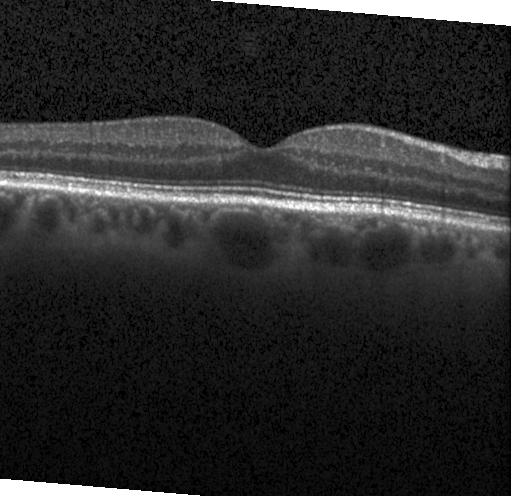

Spectral-domain OCT. Through the macula. Heidelberg Spectralis OCT system. Optical coherence tomography B-scan
Neither choroidal neovascularization, diabetic macular edema, nor drusen.